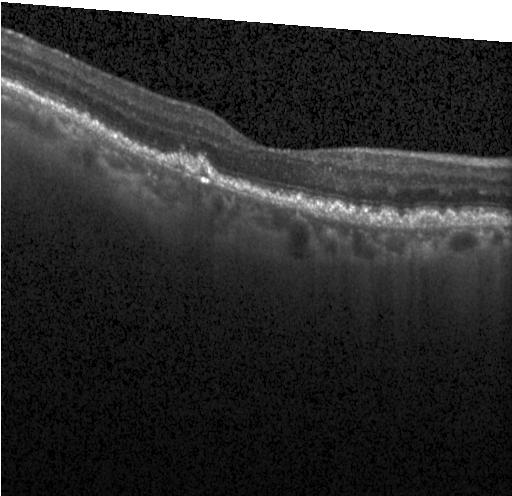

Diagnosis: drusen.